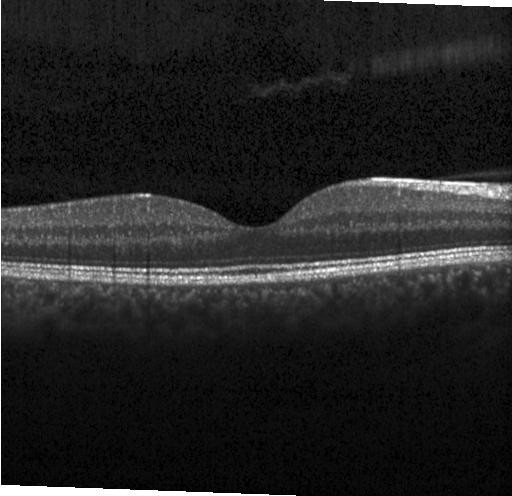
Macular OCT demonstrating no CNV, no DME, and no drusen.